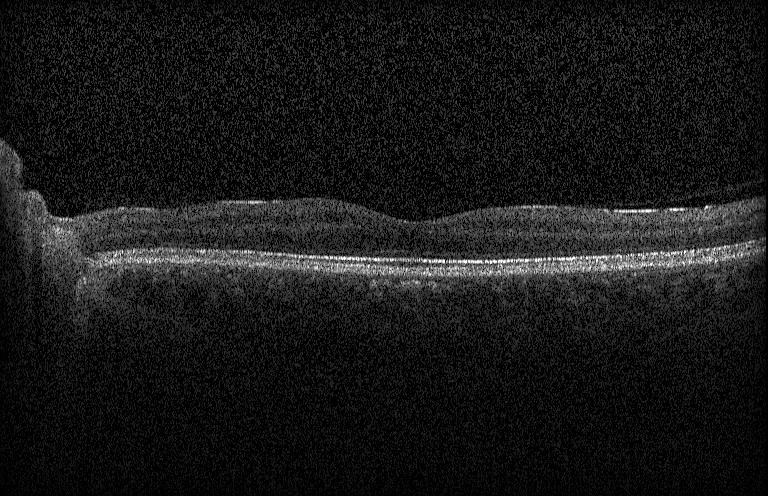

Dx: no evidence of choroidal neovascularization, diabetic macular edema, or drusen.